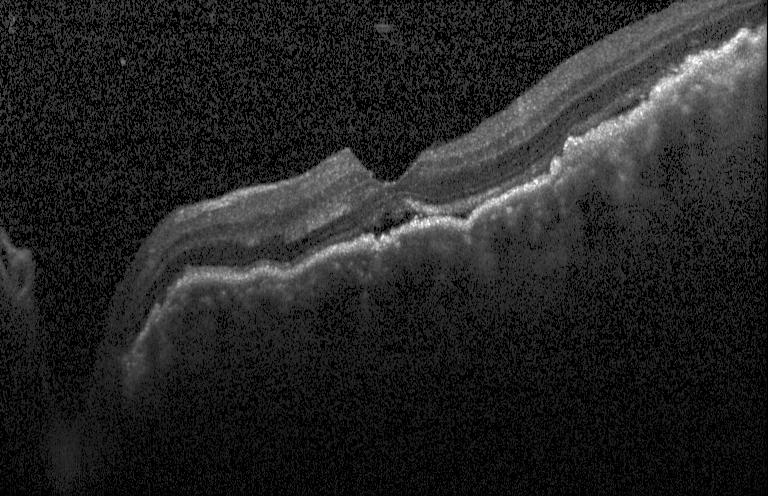
OCT B-scan · spectral-domain optical coherence tomography · macular scan.
This B-scan demonstrates CNV.